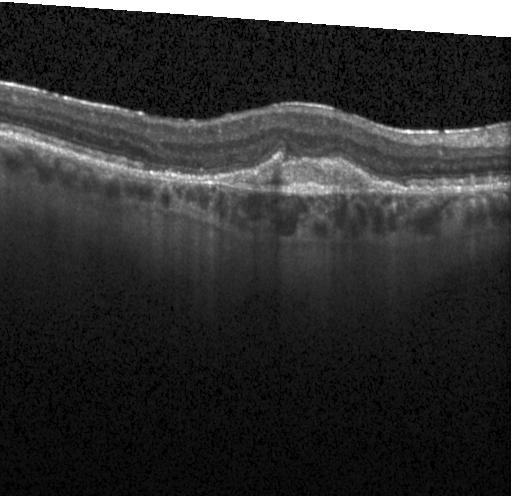

Acquired on a Heidelberg Spectralis; spectral-domain OCT; retinal OCT B-scan.
Impression: choroidal neovascularization.